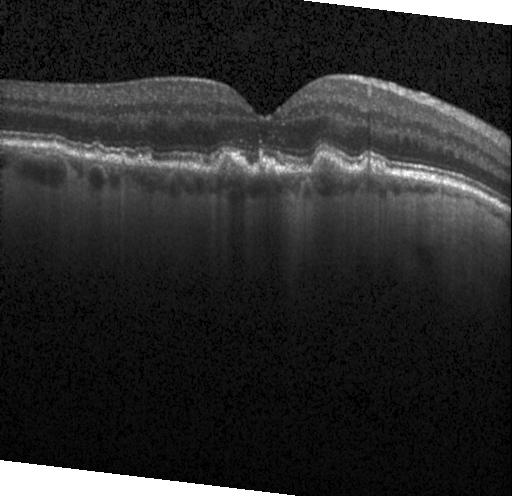

Horizontal scan through the fovea, retinal OCT cross-section
The scan shows multiple drusen.